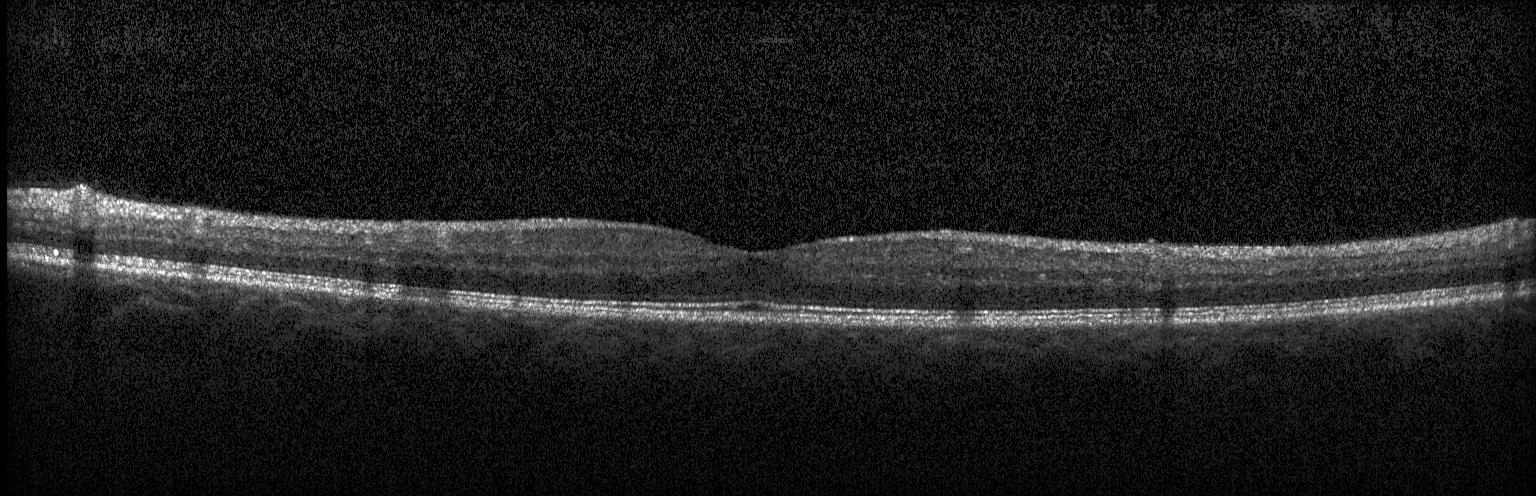 Spectral-domain OCT; centered on the fovea; Heidelberg Spectralis OCT system; retinal OCT B-scan.
Dx: neither choroidal neovascularization, diabetic macular edema, nor drusen.